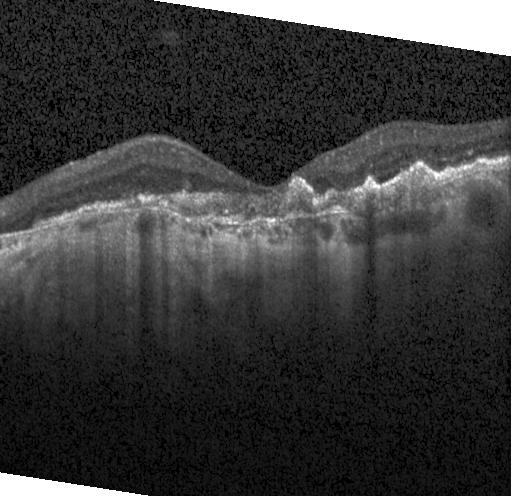

Diagnosis: a choroidal neovascular membrane.